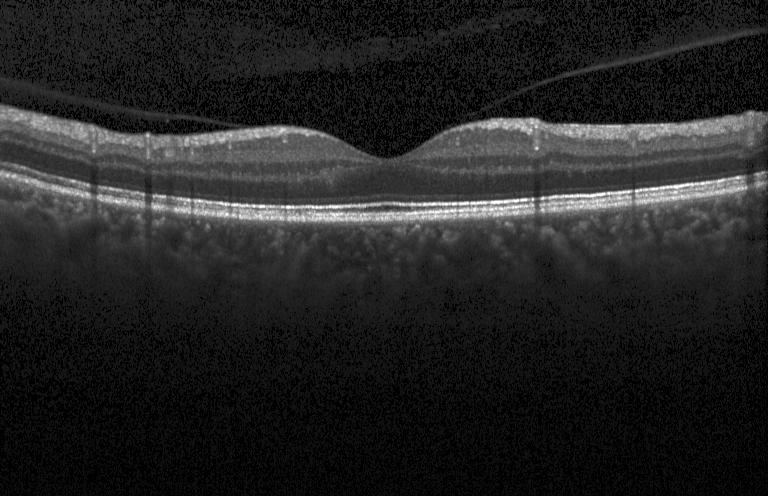

Assessment: no choroidal neovascularization, no diabetic macular edema, and no drusen.